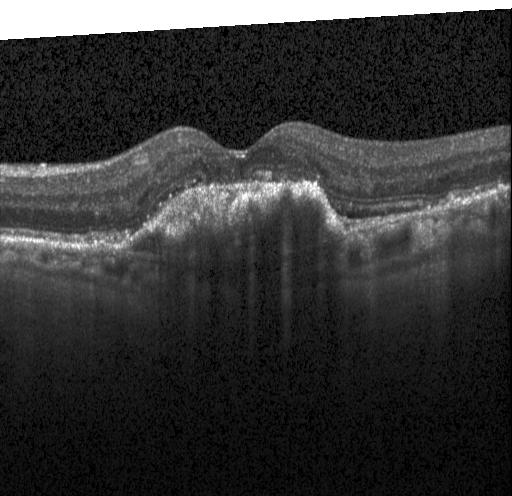 Impression: choroidal neovascularization (CNV).